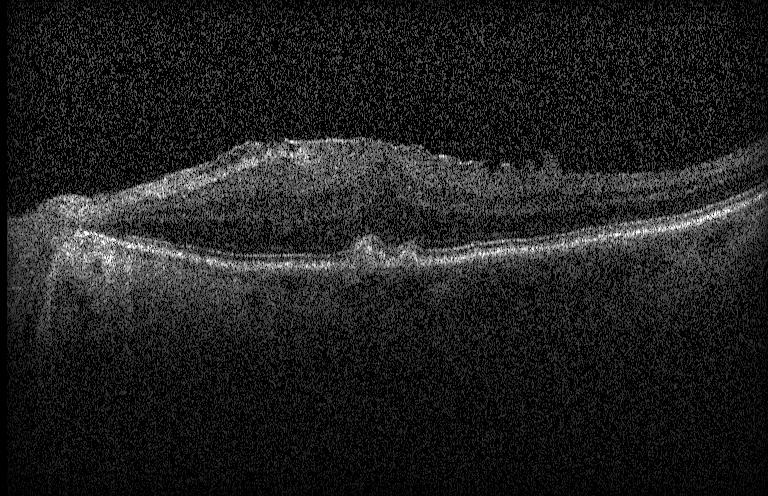

Heidelberg Spectralis; OCT B-scan; SD-OCT. OCT finding: multiple drusen.